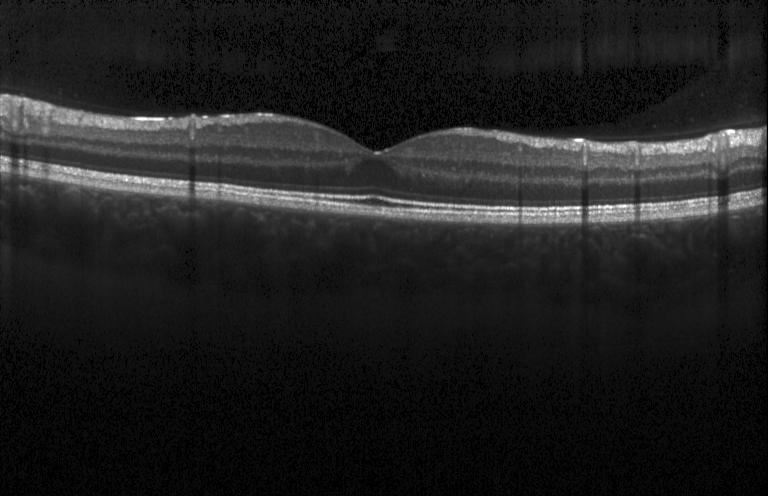
Retinal OCT cross-section. Spectral-domain optical coherence tomography. Finding: no CNV, no DME, and no drusen.